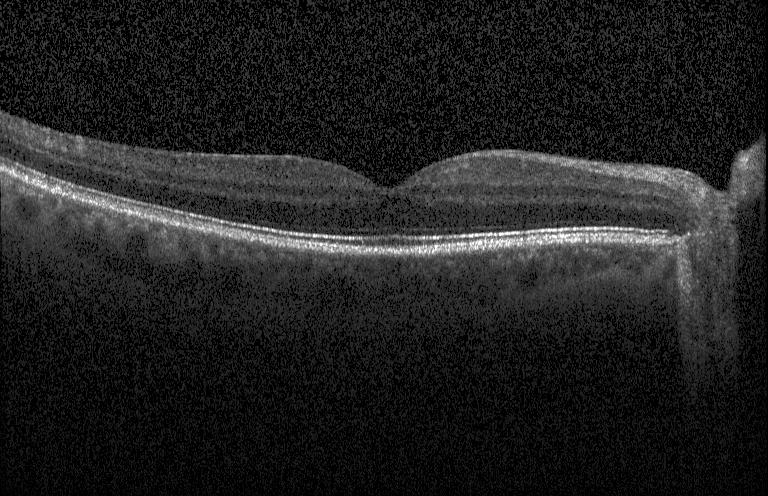

Optical coherence tomography scan
Finding: no CNV, DME, or drusen.